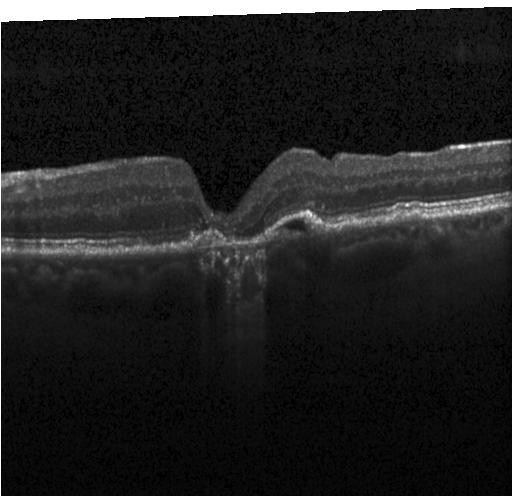 CNV.